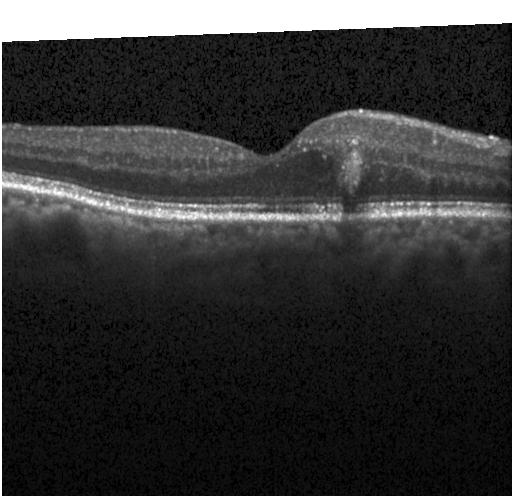
DME.